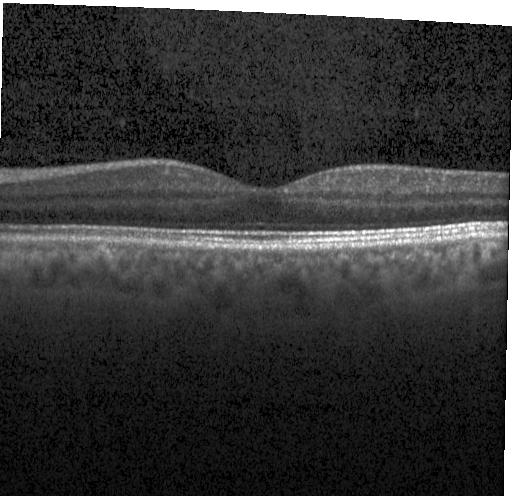

OCT B-scan. Finding: neither CNV, DME, nor drusen.